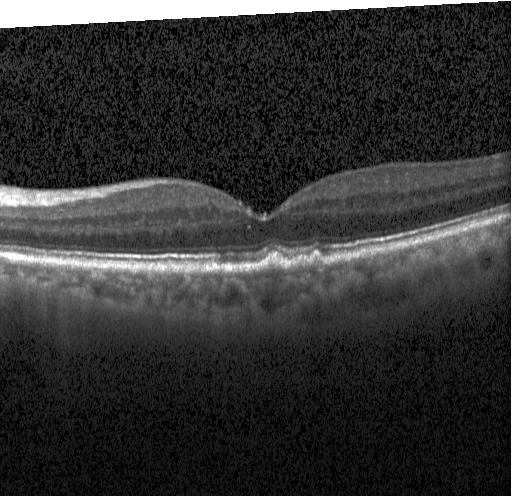

This B-scan demonstrates sub-RPE drusenoid deposits.